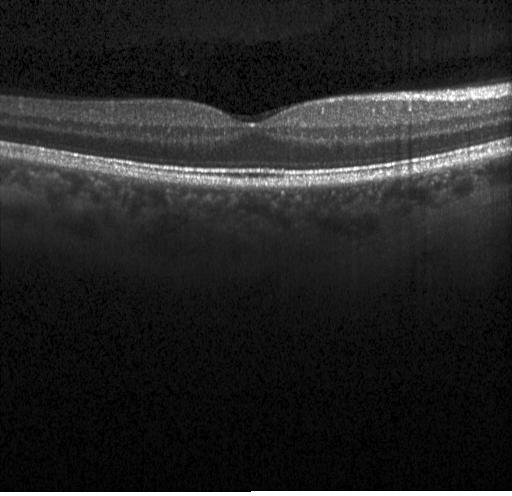

Optical coherence tomography B-scan — Finding: no evidence of choroidal neovascularization, diabetic macular edema, or drusen.